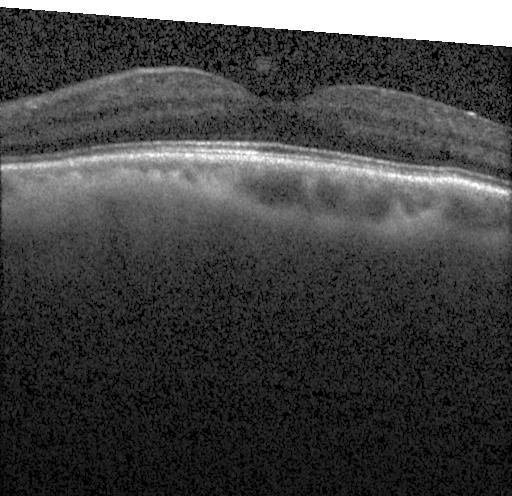
Horizontal scan through the fovea, OCT B-scan, Heidelberg Spectralis OCT system
Finding: no choroidal neovascularization, diabetic macular edema, or drusen.